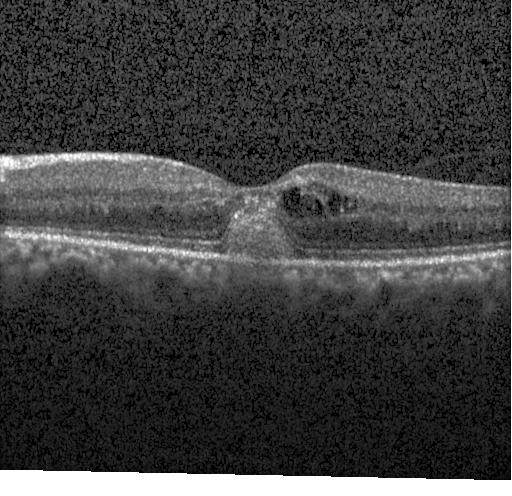 OCT finding: CNV.